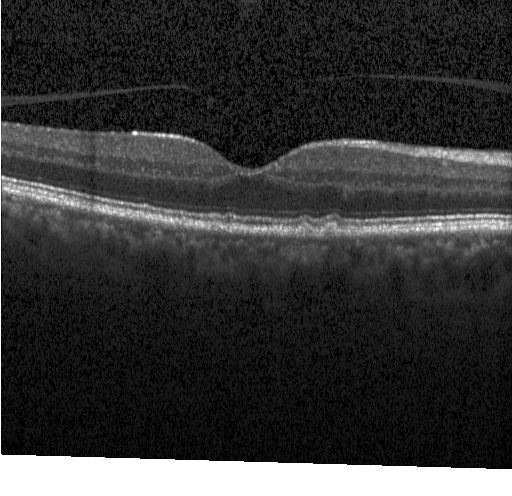 Diagnosis: drusen.